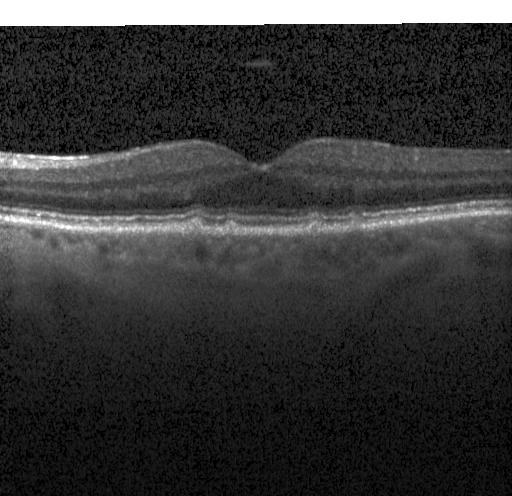 Acquired on a Heidelberg Spectralis, retinal OCT cross-section, centered on the fovea — This B-scan demonstrates sub-RPE drusenoid deposits.